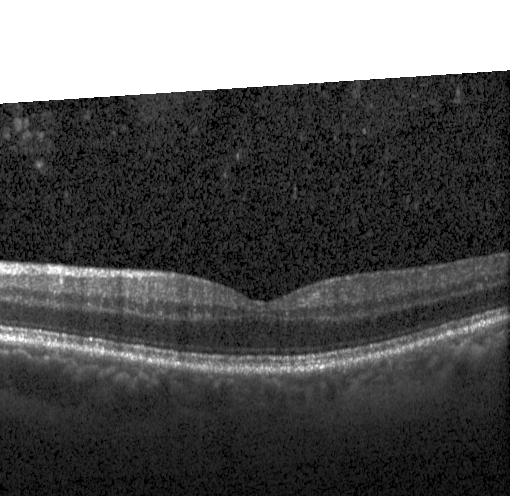 Spectral-domain OCT. Optical coherence tomography scan.
This B-scan demonstrates no choroidal neovascularization, diabetic macular edema, or drusen.